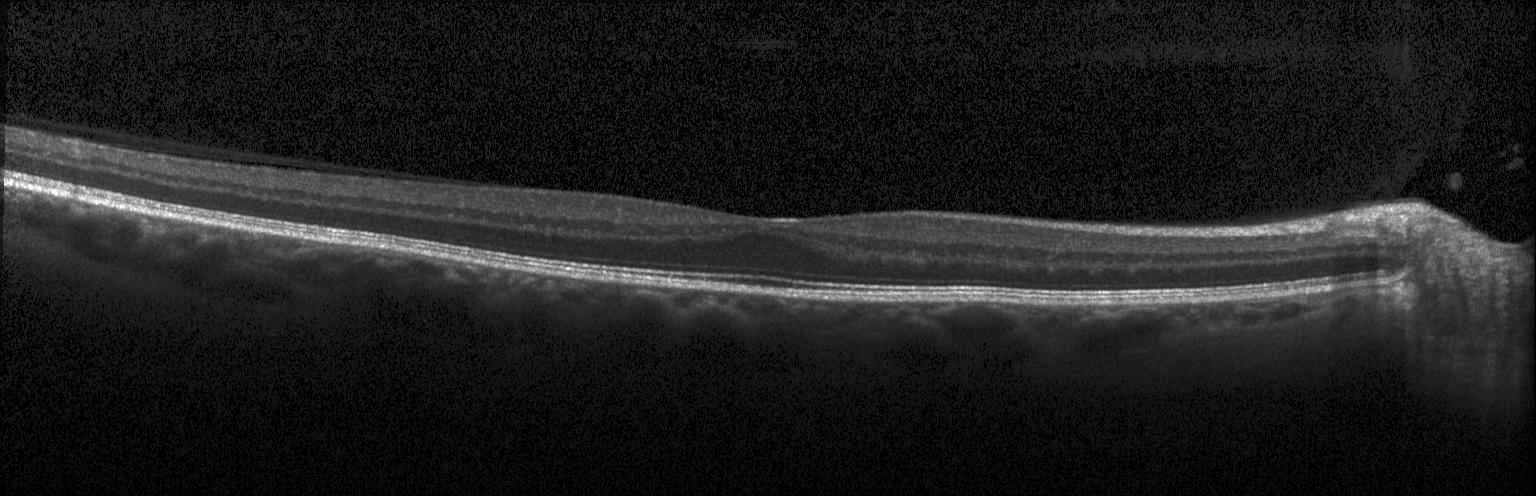 Retinal OCT cross-section showing no evidence of choroidal neovascularization, diabetic macular edema, or drusen.